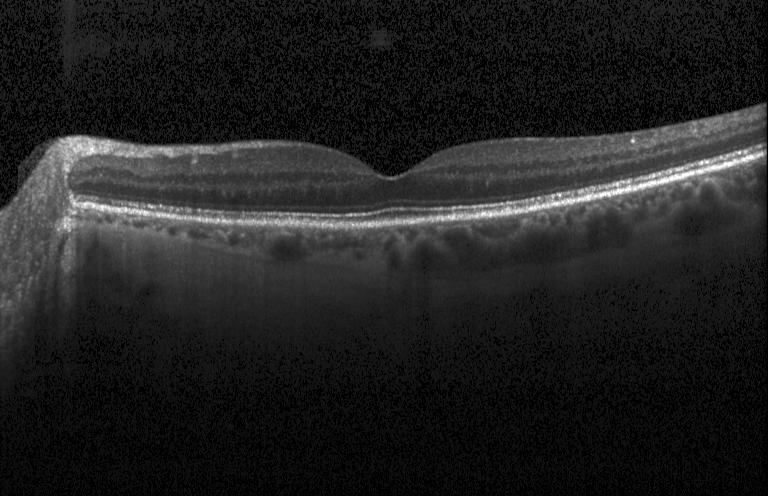 Diagnosis: no evidence of choroidal neovascularization, diabetic macular edema, or drusen.